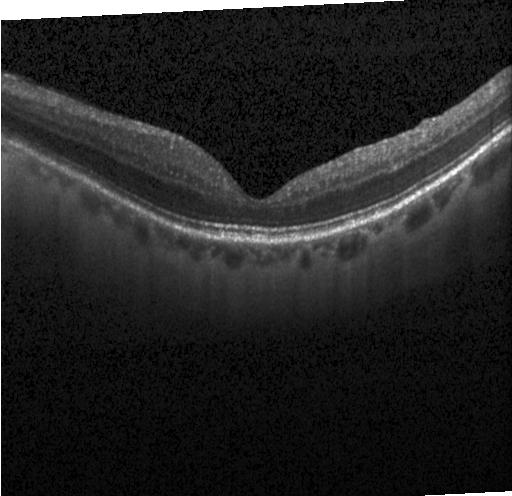 Optical coherence tomography B-scan; acquired on a Heidelberg Spectralis; horizontal scan through the fovea; spectral-domain optical coherence tomography.
Assessment: no evidence of choroidal neovascularization, diabetic macular edema, or drusen.